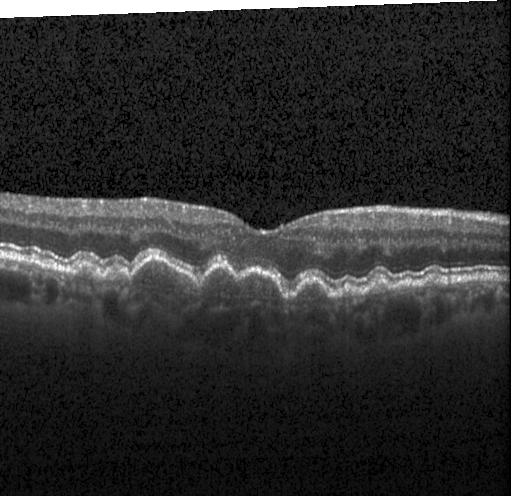 OCT B-scan. Through the macula. SD-OCT. Finding: multiple drusen.